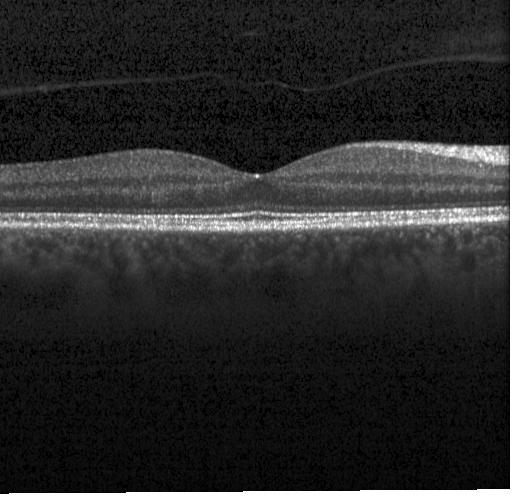
OCT B-scan; spectral-domain OCT; acquired on a Heidelberg Spectralis
Macular OCT: neither choroidal neovascularization, diabetic macular edema, nor drusen.